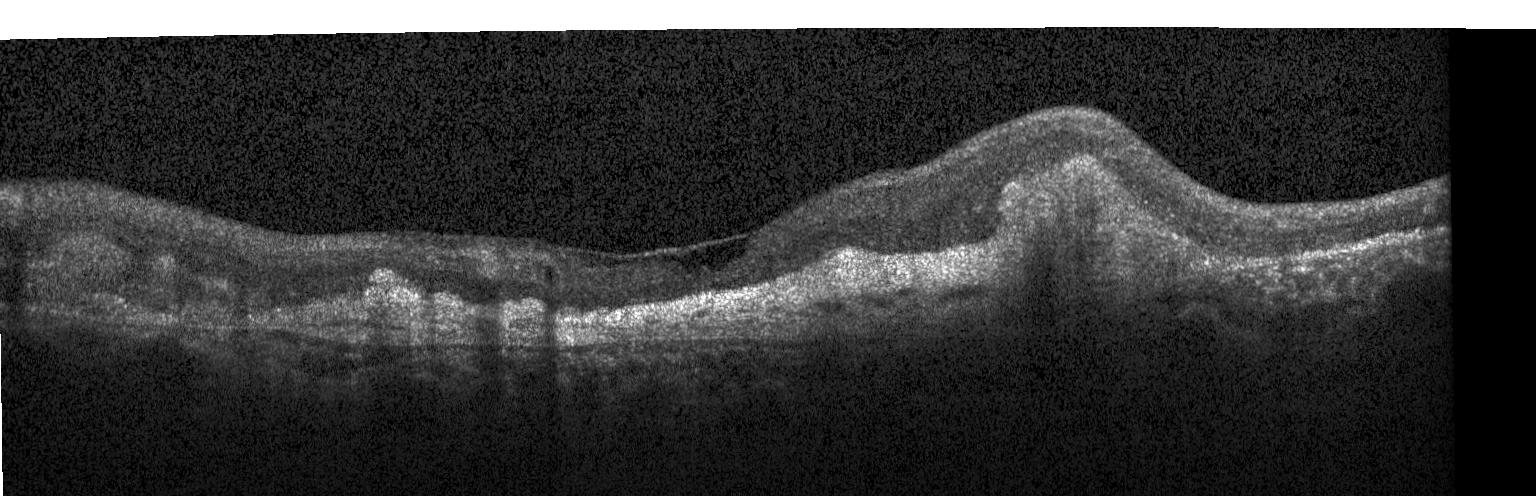
This B-scan demonstrates a choroidal neovascular membrane.